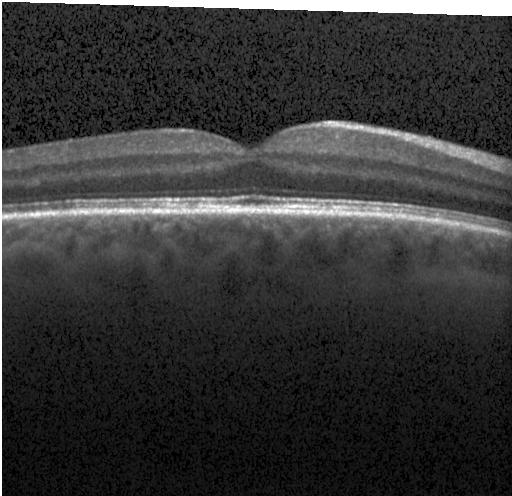 OCT line scan · spectral-domain optical coherence tomography · horizontal scan through the fovea
The scan shows no choroidal neovascularization, no diabetic macular edema, and no drusen.